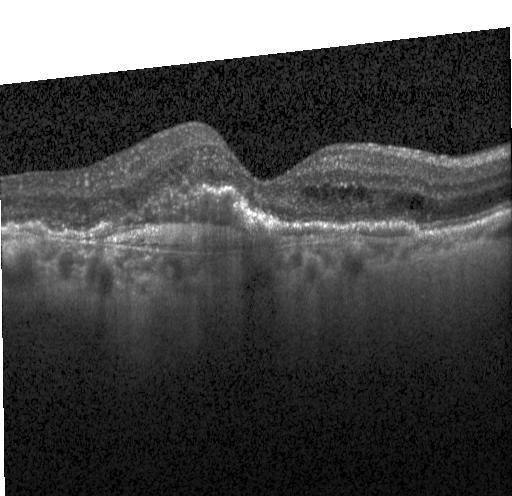

Retinal OCT cross-section showing a choroidal neovascular membrane.